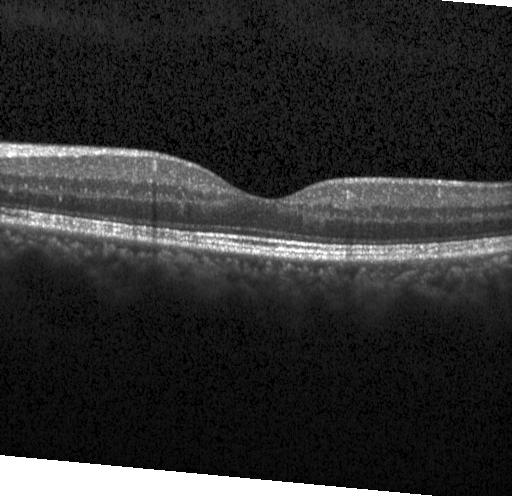
Optical coherence tomography B-scan. Centered on the fovea. Spectral-domain optical coherence tomography. Heidelberg Spectralis.
Impression: no choroidal neovascularization, diabetic macular edema, or drusen.